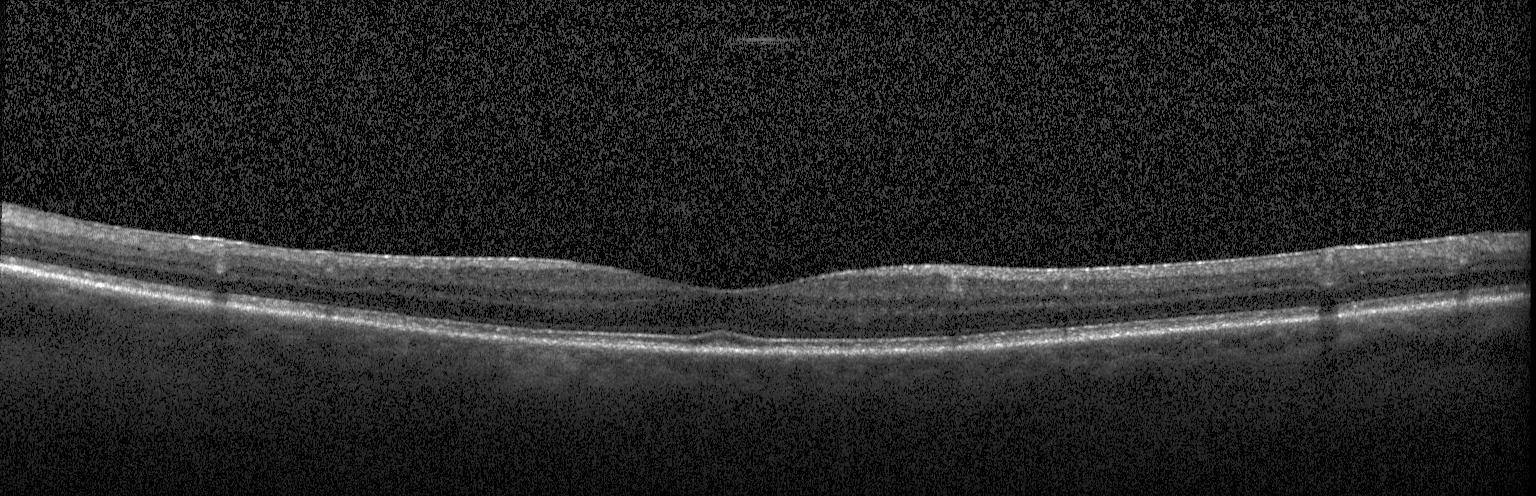 Optical coherence tomography scan, macular scan, Heidelberg Spectralis OCT system, SD-OCT — Diagnosis: no evidence of CNV, DME, or drusen.